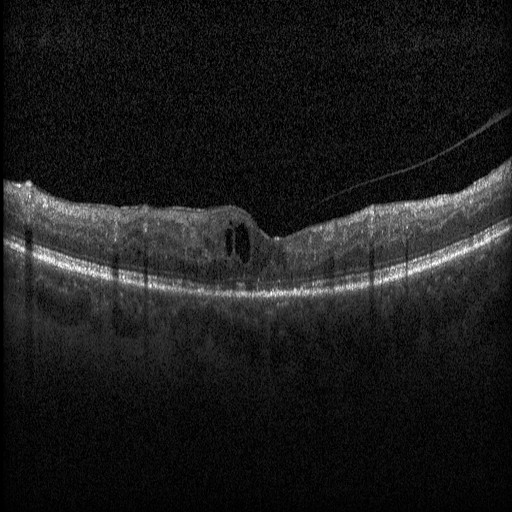
Optical coherence tomography B-scan. Impression: diabetic macular edema.